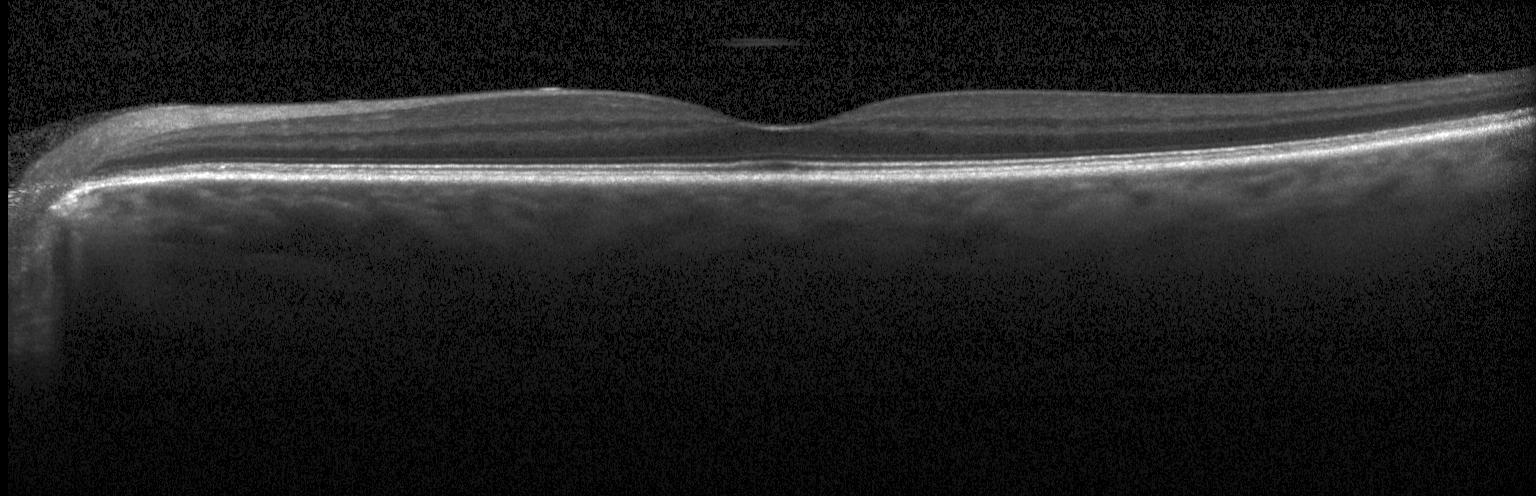 Impression: neither choroidal neovascularization, diabetic macular edema, nor drusen.